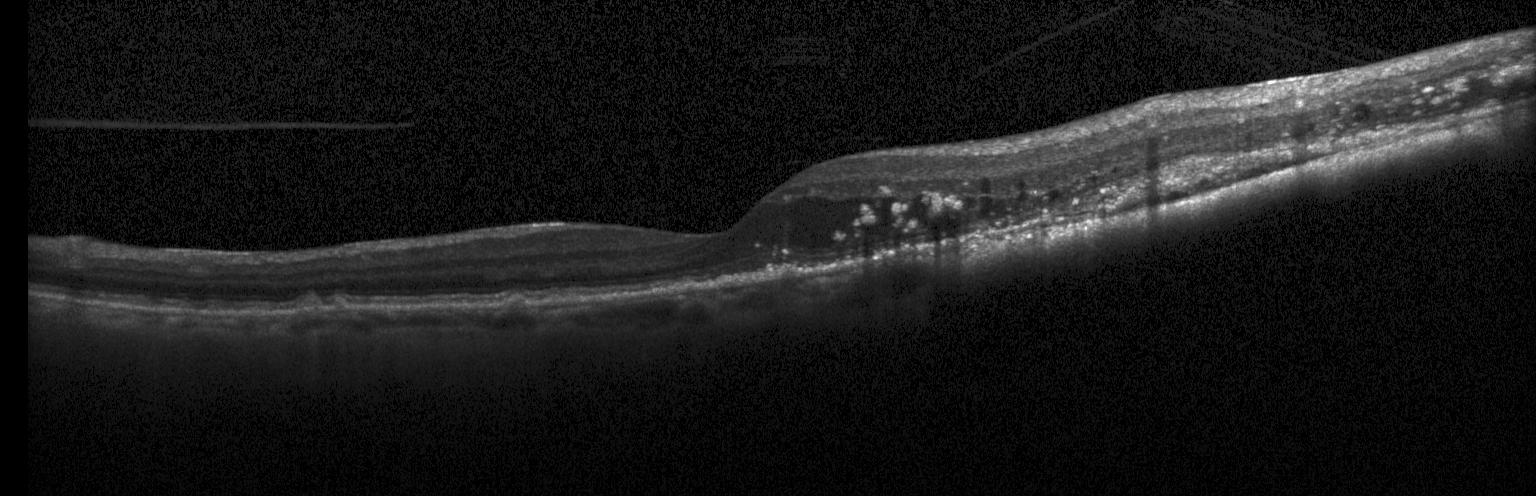

Optical coherence tomography scan — This B-scan demonstrates CNV.